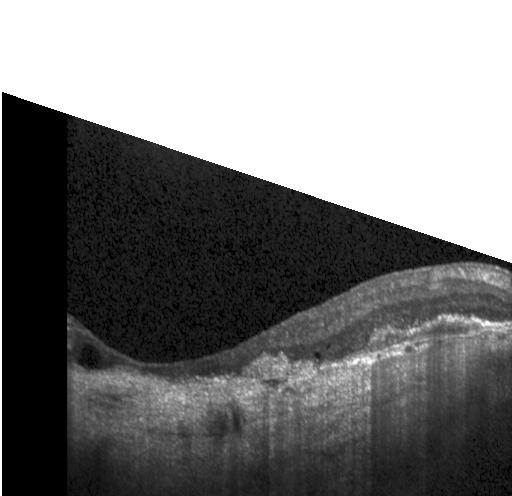 Macular OCT: choroidal neovascularization.